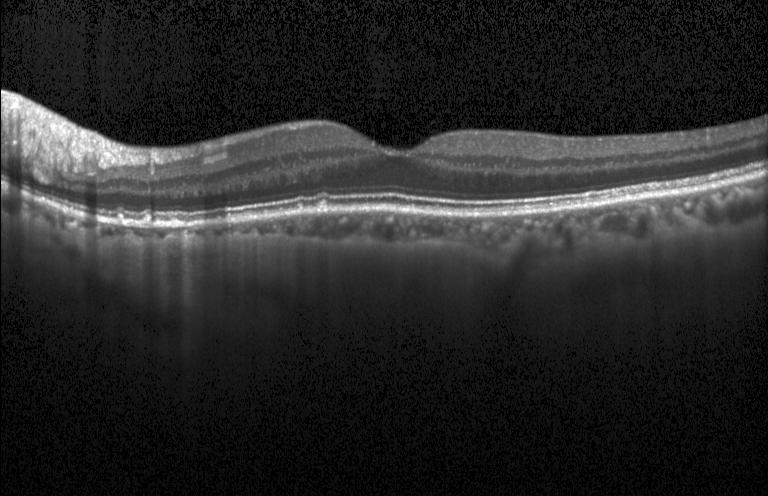 Instrument: Heidelberg Spectralis, optical coherence tomography B-scan — This B-scan demonstrates drusen.